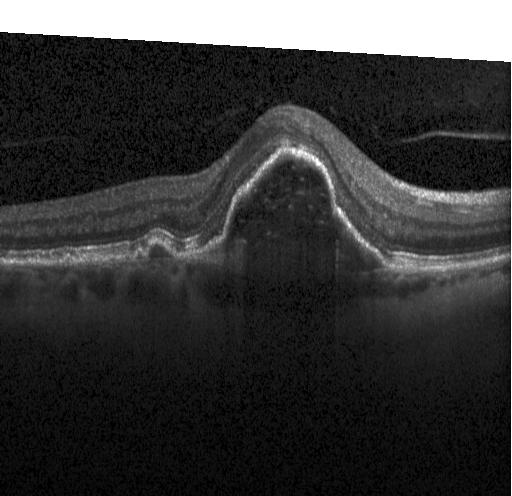
Horizontal scan through the fovea, retinal OCT B-scan, spectral-domain OCT
OCT finding: choroidal neovascularization.